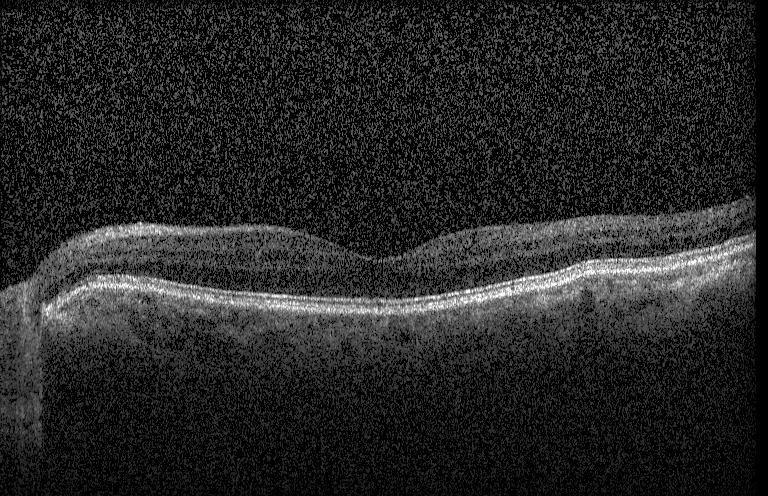 Retinal OCT cross-section showing no evidence of choroidal neovascularization, diabetic macular edema, or drusen.